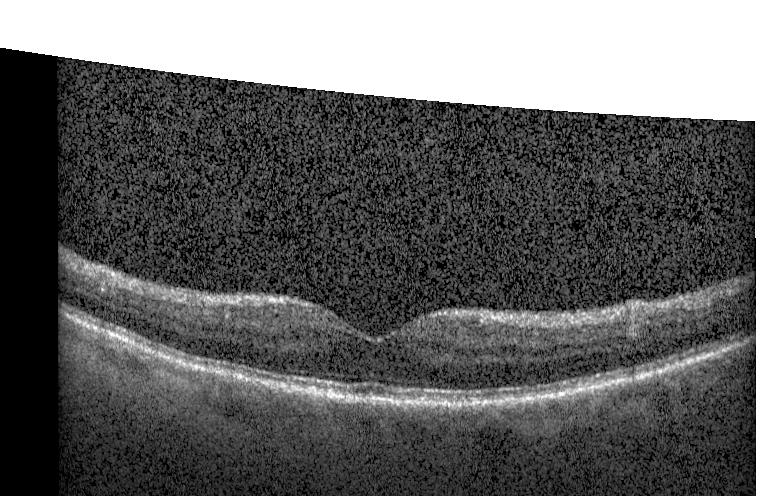 Finding: no choroidal neovascularization, no diabetic macular edema, and no drusen.